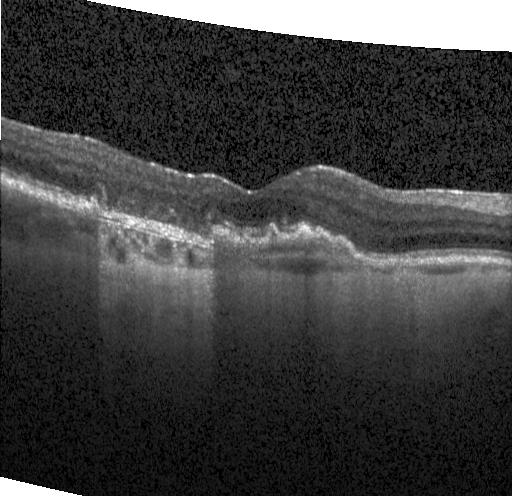 Optical coherence tomography B-scan; centered on the fovea; instrument: Heidelberg Spectralis; spectral-domain optical coherence tomography
The scan shows a choroidal neovascular membrane.